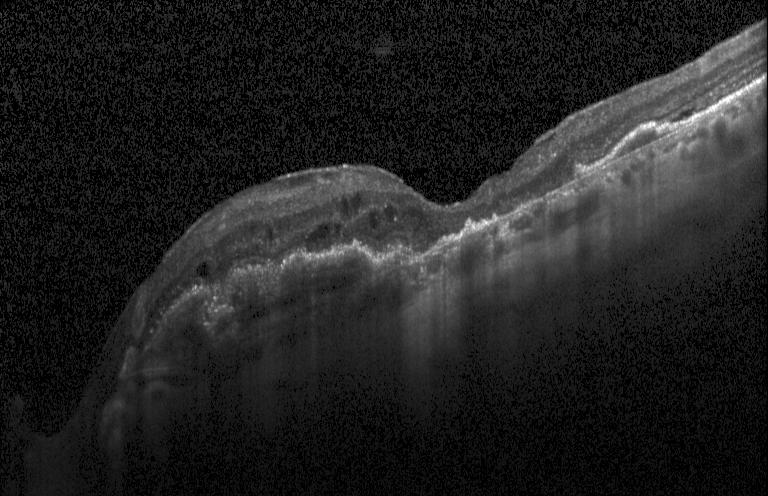
The scan shows a choroidal neovascular membrane.